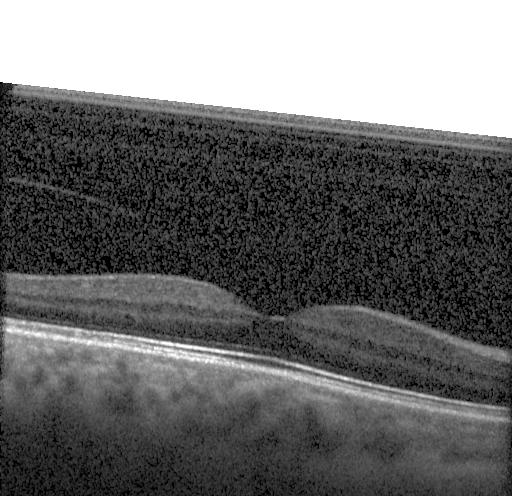 Optical coherence tomography B-scan. Diagnosis: no choroidal neovascularization, no diabetic macular edema, and no drusen.